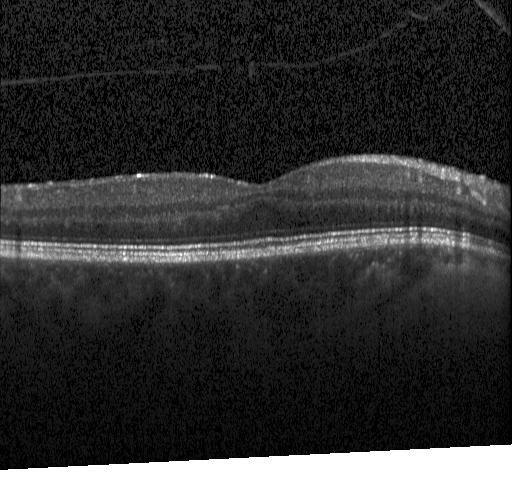
Acquired on a Heidelberg Spectralis, spectral-domain OCT, OCT B-scan
Impression: no choroidal neovascularization, no diabetic macular edema, and no drusen.